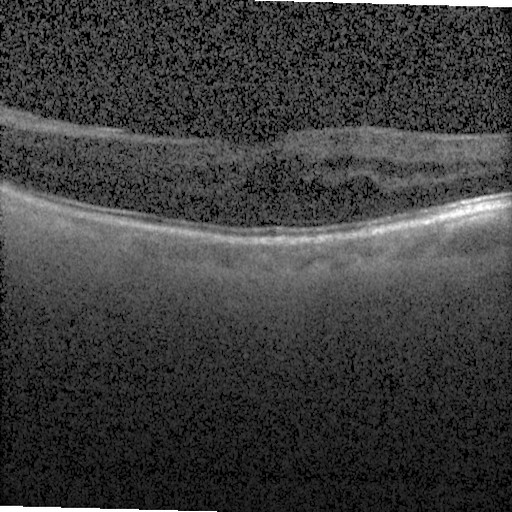 Retinal OCT cross-section. Assessment: DME.